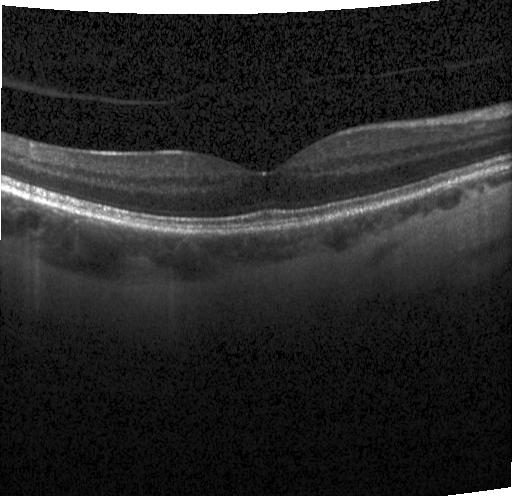

Acquired on a Heidelberg Spectralis; optical coherence tomography scan; horizontal scan through the fovea; spectral-domain OCT. Macular OCT: no choroidal neovascularization, diabetic macular edema, or drusen.